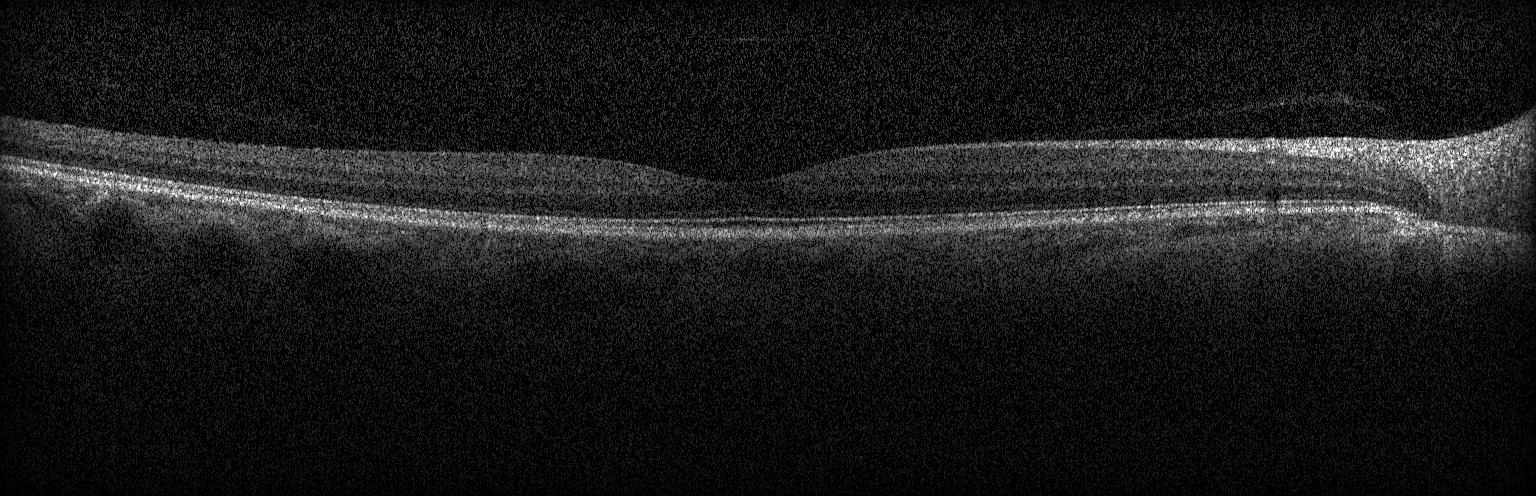

OCT B-scan.
Finding: no choroidal neovascularization, no diabetic macular edema, and no drusen.